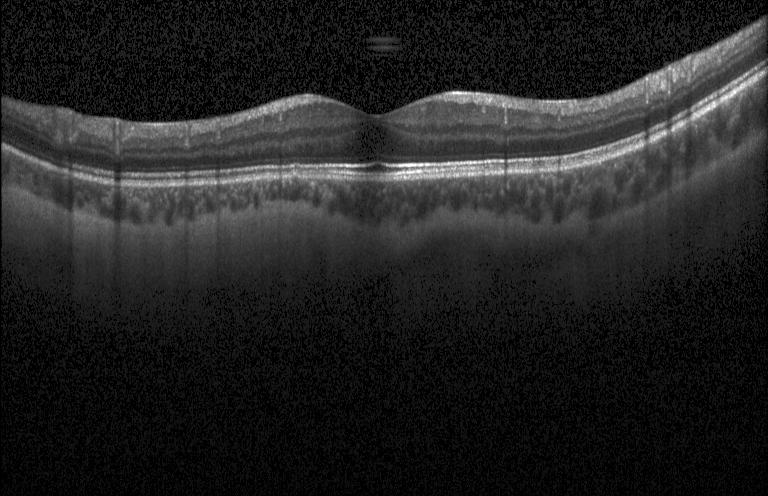
Optical coherence tomography scan
The scan shows no choroidal neovascularization, no diabetic macular edema, and no drusen.